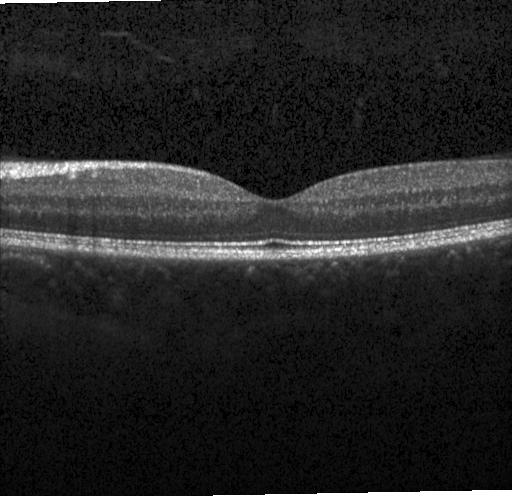

Neither CNV, DME, nor drusen.